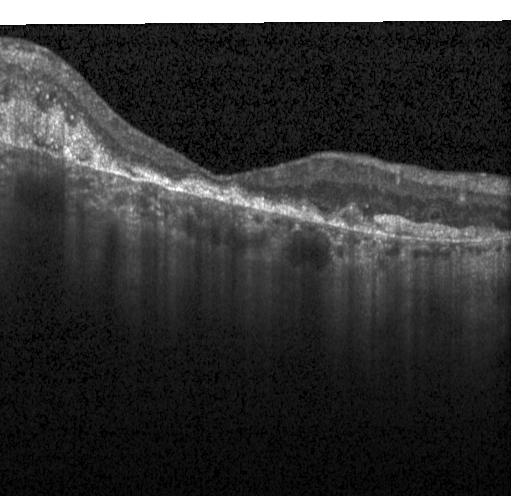

Spectral-domain optical coherence tomography · optical coherence tomography scan · Heidelberg Spectralis · centered on the fovea.
Impression: a choroidal neovascular membrane.